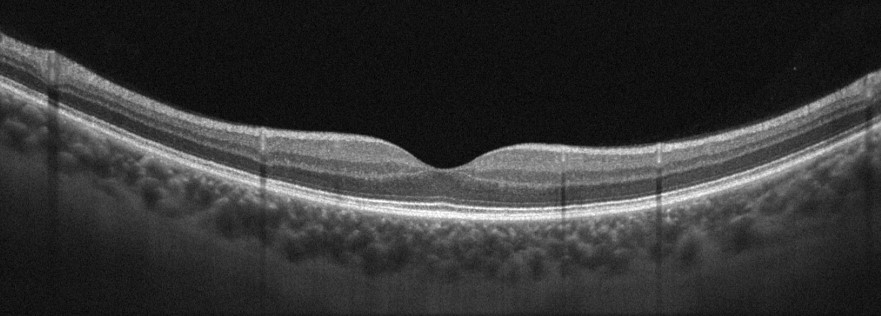
Optical coherence tomography B-scan. Instrument: Optovue Avanti RTVue XR. Macular scan.
Impression: no AMD, DME, ERM, RAO, RVO, or VID.